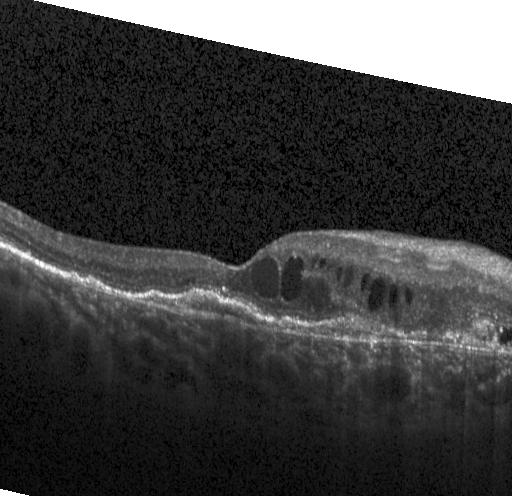 Retinal OCT cross-section · Heidelberg Spectralis
Assessment: choroidal neovascularization (CNV).